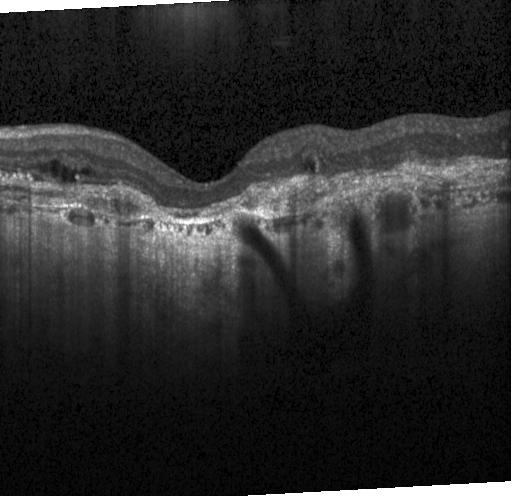 OCT line scan
Choroidal neovascularization (CNV).